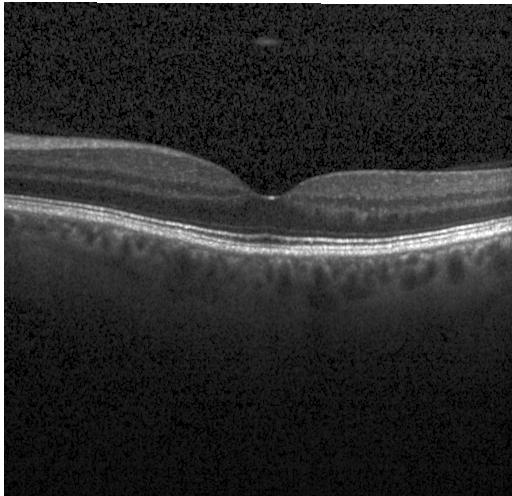
OCT B-scan · instrument: Heidelberg Spectralis · SD-OCT · fovea-centered.
OCT finding: neither CNV, DME, nor drusen.